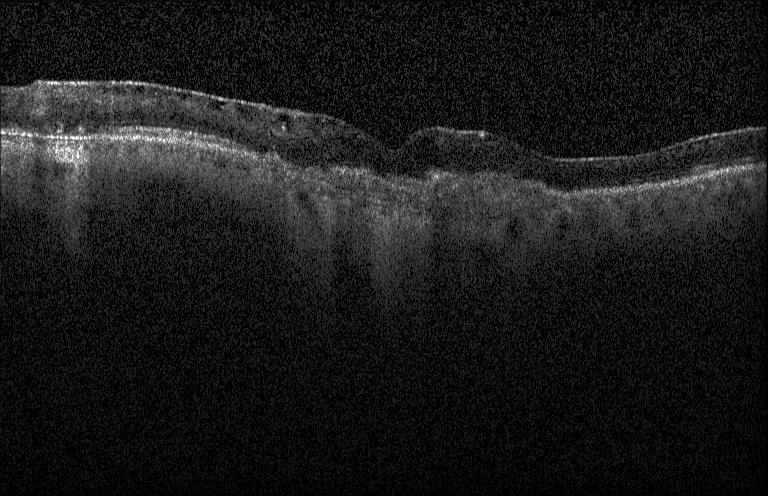 OCT line scan · Heidelberg Spectralis · spectral-domain optical coherence tomography. Diagnosis: choroidal neovascularization.